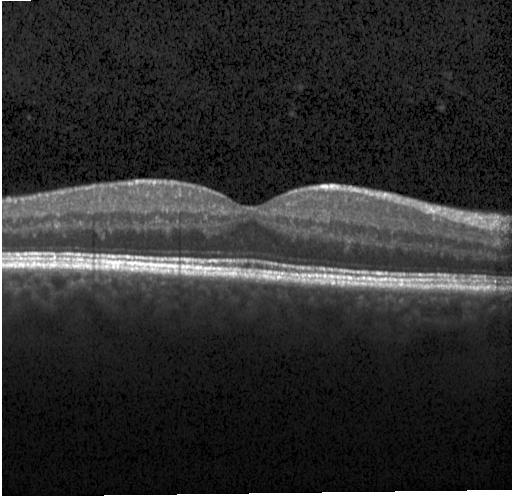
Impression: no CNV, no DME, and no drusen.